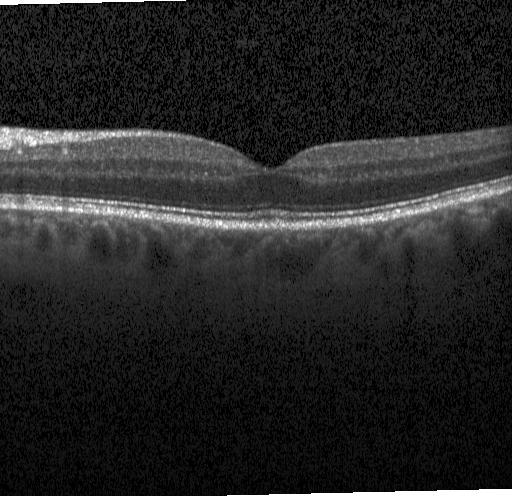 Horizontal scan through the fovea. Heidelberg Spectralis OCT system. Optical coherence tomography scan. Spectral-domain OCT
Assessment: no choroidal neovascularization, diabetic macular edema, or drusen.